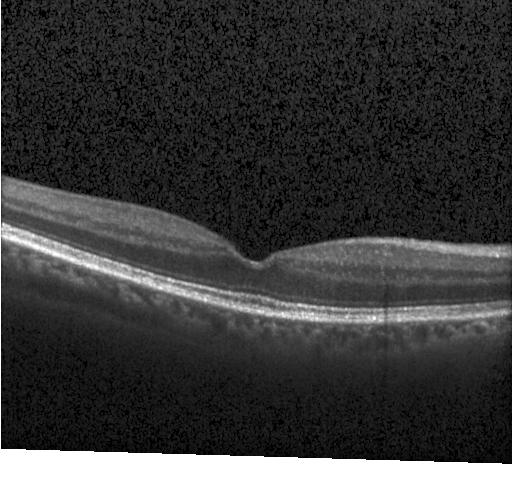
Centered on the fovea · optical coherence tomography B-scan. This B-scan demonstrates no choroidal neovascularization, diabetic macular edema, or drusen.